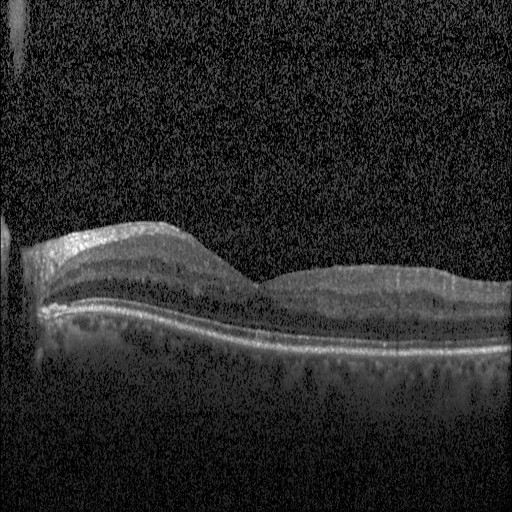 OCT line scan. Diagnosis: diabetic macular edema (DME).